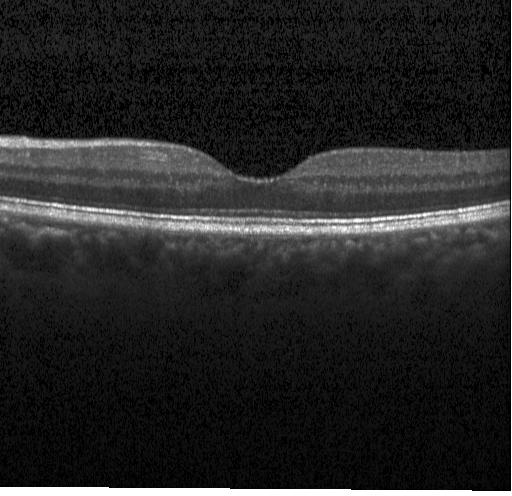
Acquired on a Heidelberg Spectralis. Retinal OCT cross-section. SD-OCT. Horizontal scan through the fovea — Macular OCT: no choroidal neovascularization, no diabetic macular edema, and no drusen.